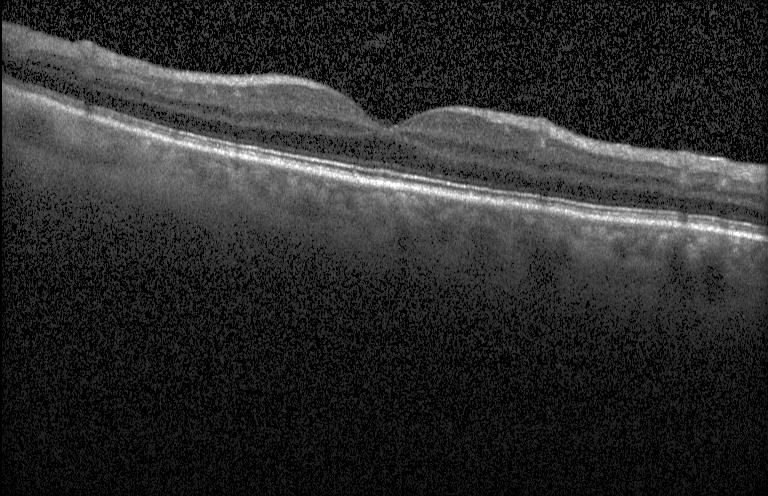
Impression: no evidence of choroidal neovascularization, diabetic macular edema, or drusen.